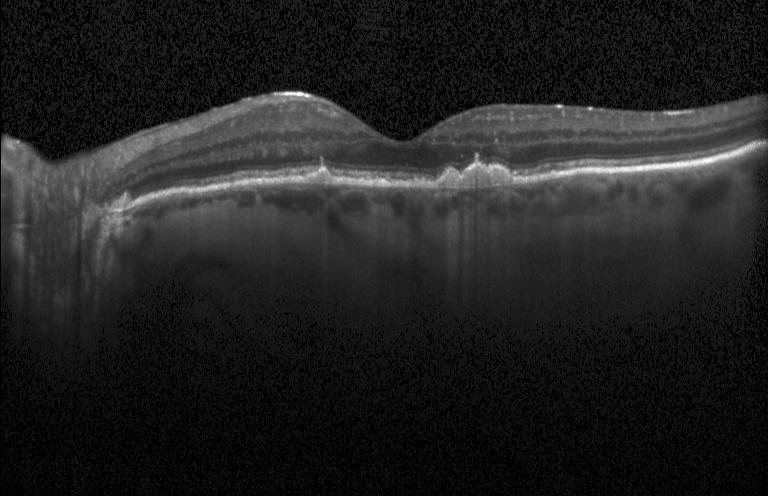

Retinal OCT cross-section. Diagnosis: drusen.